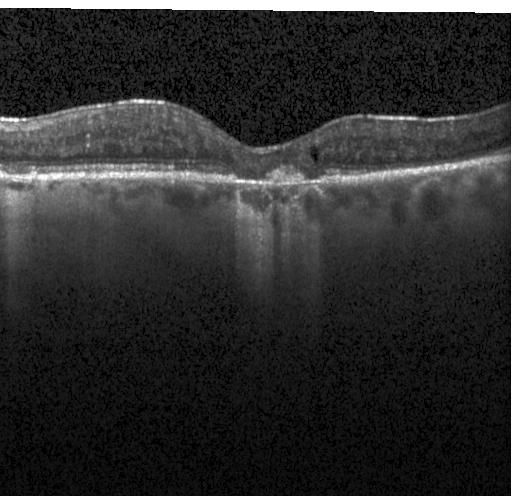 Acquired on a Heidelberg Spectralis, retinal OCT cross-section, fovea-centered
Assessment: a choroidal neovascular membrane.